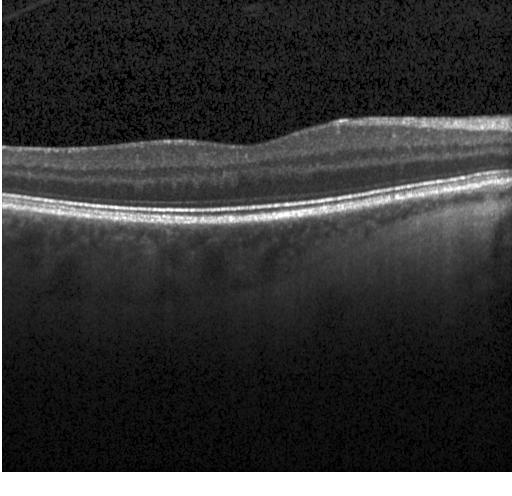 Retinal OCT cross-section showing no choroidal neovascularization, no diabetic macular edema, and no drusen.